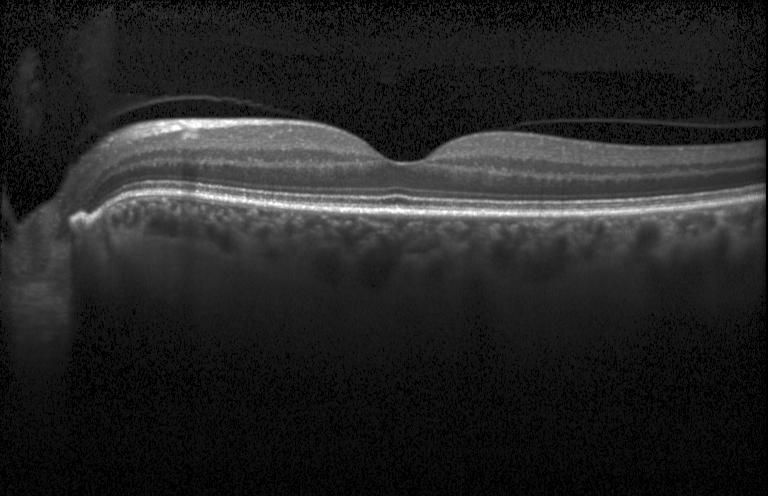
Assessment: neither CNV, DME, nor drusen.